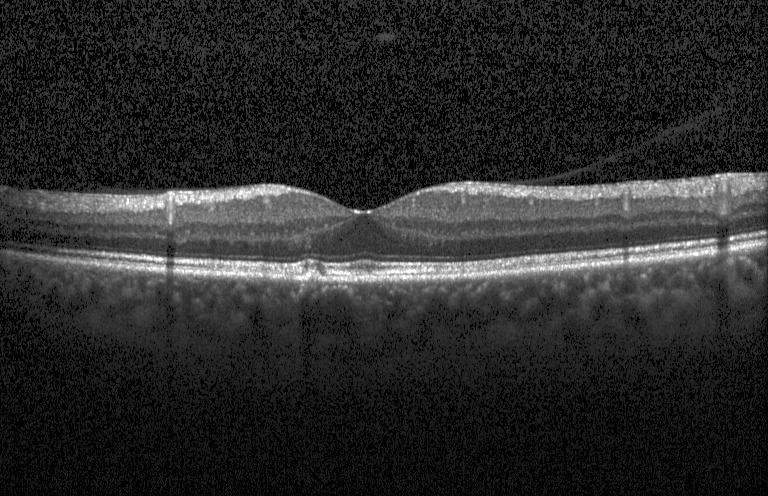 Heidelberg Spectralis. Centered on the fovea. Optical coherence tomography B-scan — Impression: neither CNV, DME, nor drusen.